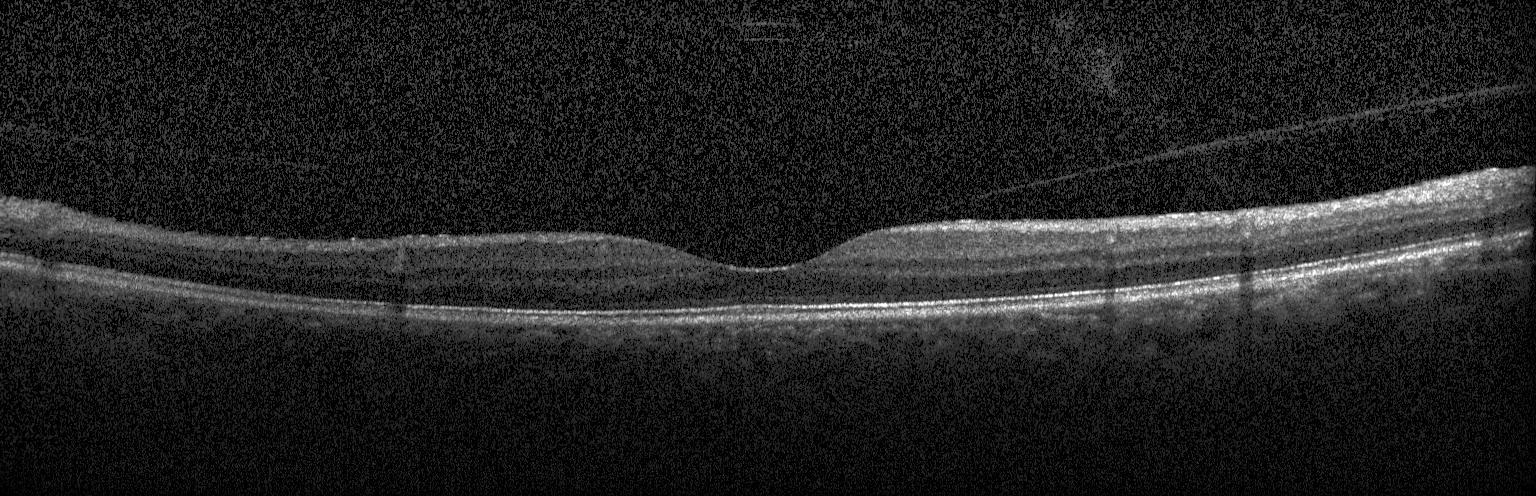
Horizontal scan through the fovea · retinal OCT cross-section. Diagnosis: no evidence of choroidal neovascularization, diabetic macular edema, or drusen.